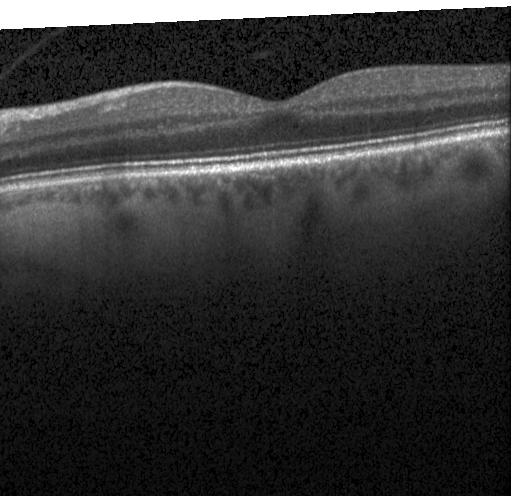
Centered on the fovea; retinal OCT B-scan; spectral-domain optical coherence tomography; instrument: Heidelberg Spectralis. Finding: neither choroidal neovascularization, diabetic macular edema, nor drusen.